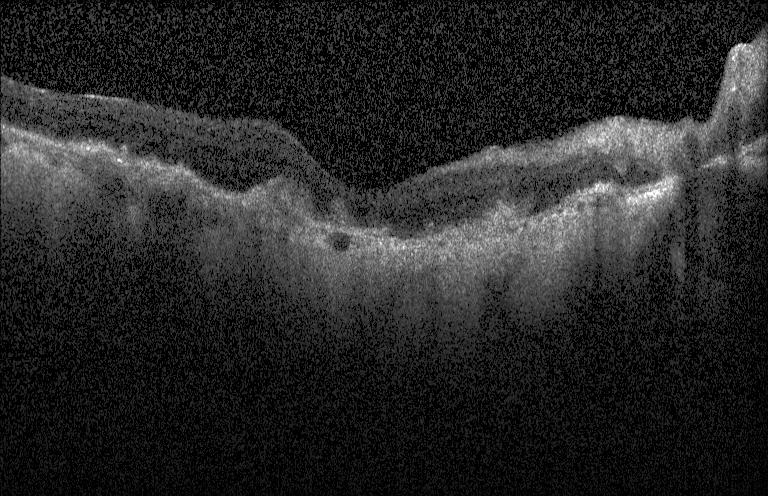 OCT B-scan showing CNV.